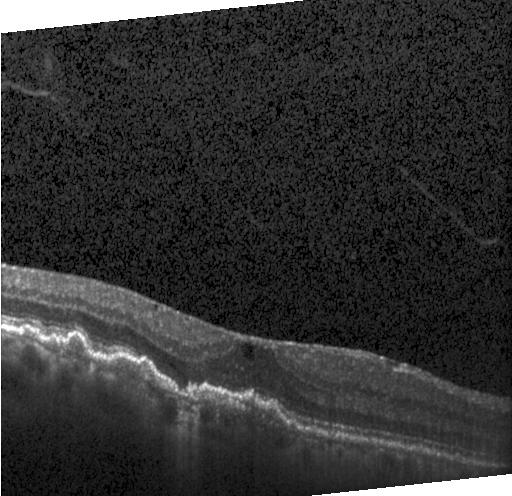 A choroidal neovascular membrane.